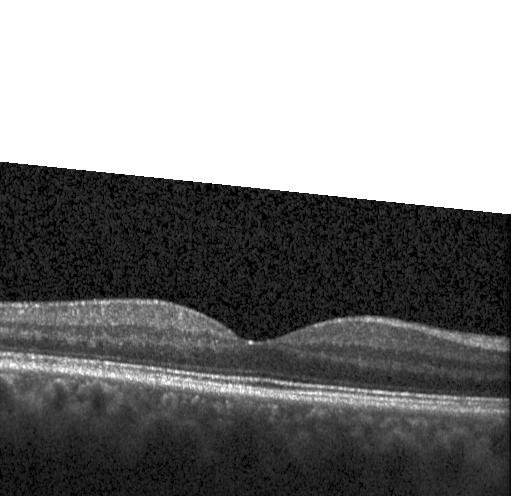
The scan shows no evidence of CNV, DME, or drusen.